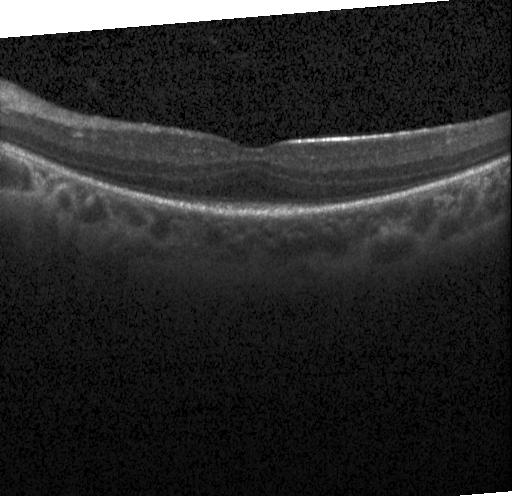

Fovea-centered. SD-OCT. Heidelberg Spectralis OCT system. Retinal OCT B-scan.
Finding: no choroidal neovascularization, no diabetic macular edema, and no drusen.